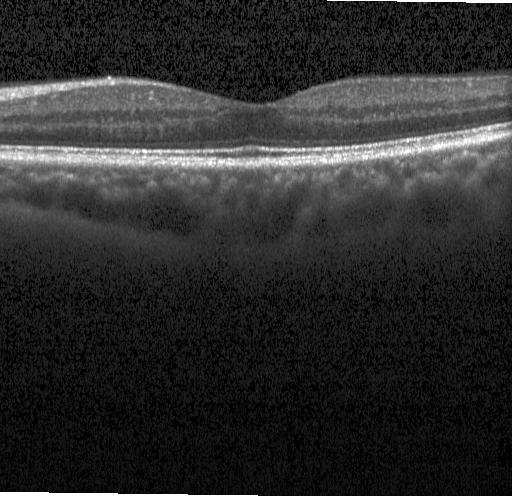

Optical coherence tomography B-scan.
Macular OCT: no CNV, no DME, and no drusen.